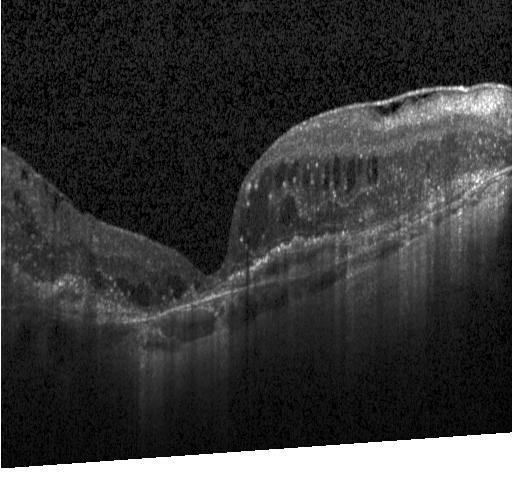
Finding: choroidal neovascularization (CNV).